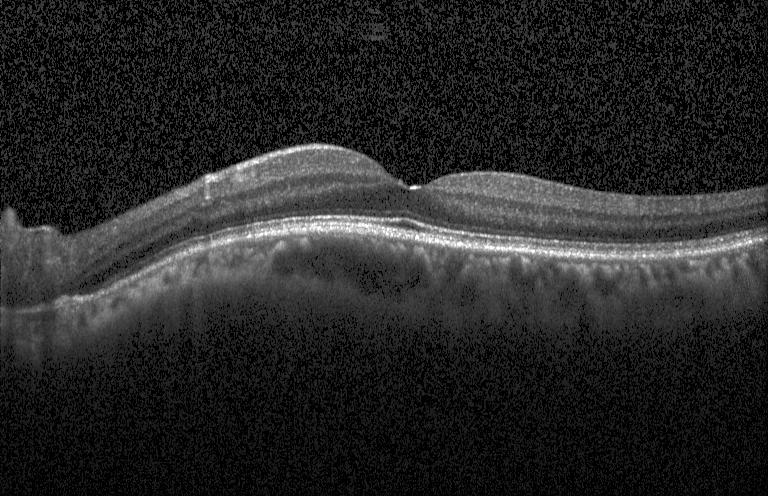 Diagnosis: no evidence of choroidal neovascularization, diabetic macular edema, or drusen.